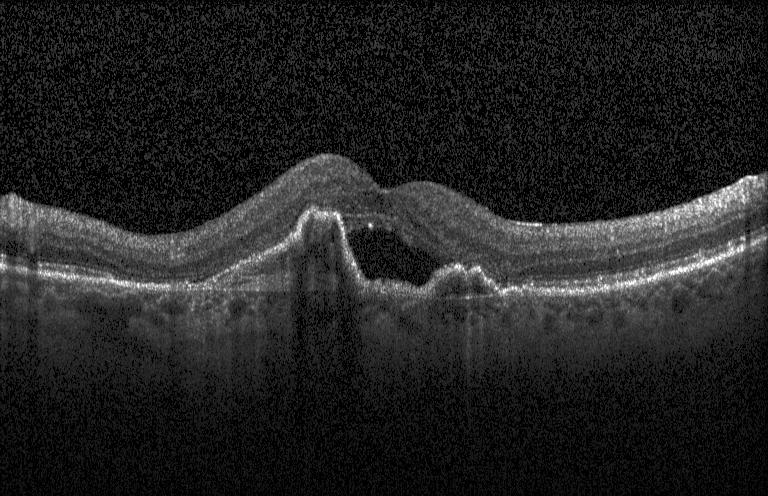

Impression: a choroidal neovascular membrane.